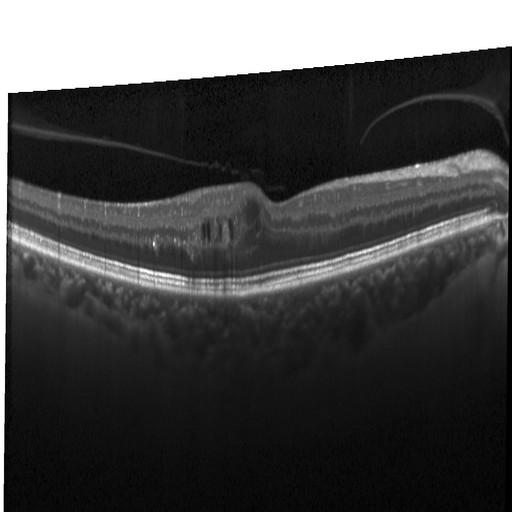
Retinal OCT cross-section; spectral-domain optical coherence tomography; macular scan
The scan shows diabetic macular edema.